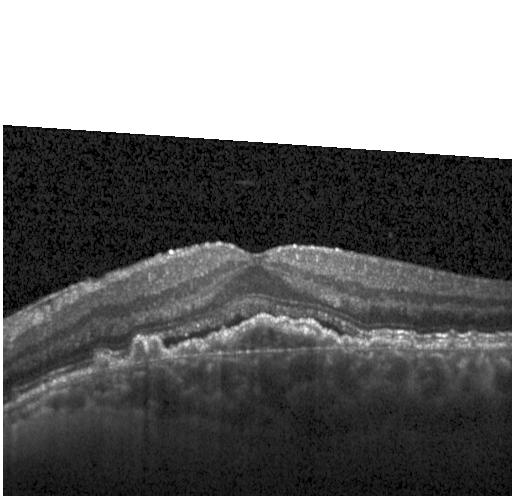
OCT B-scan showing a choroidal neovascular membrane.